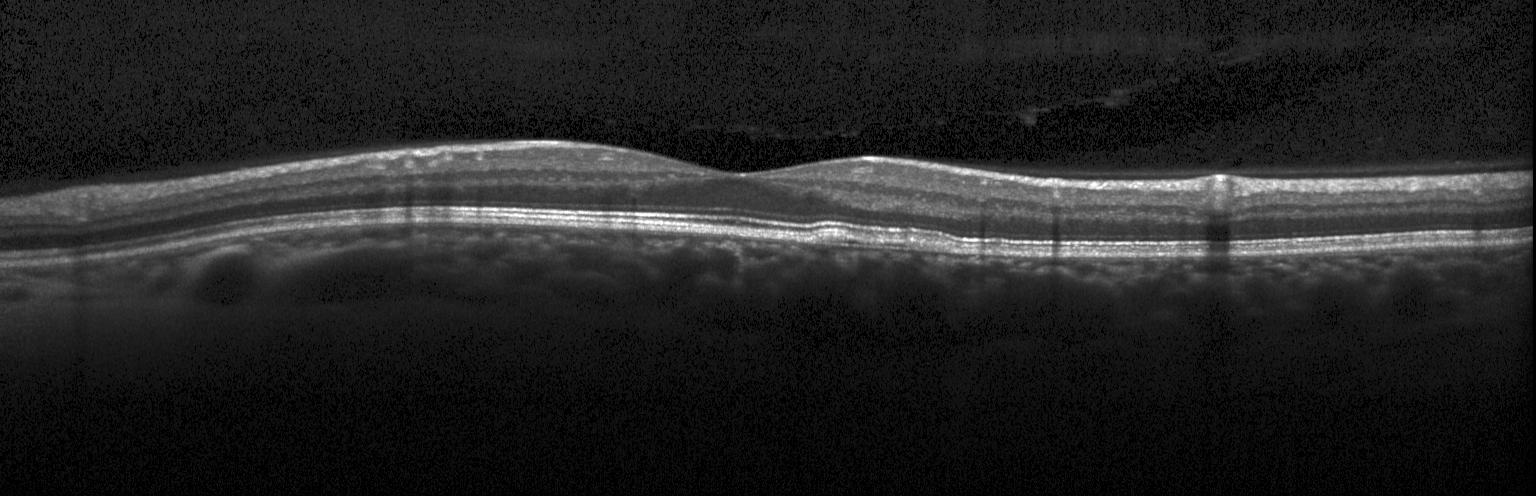

Horizontal scan through the fovea · optical coherence tomography B-scan. Dx: CNV.